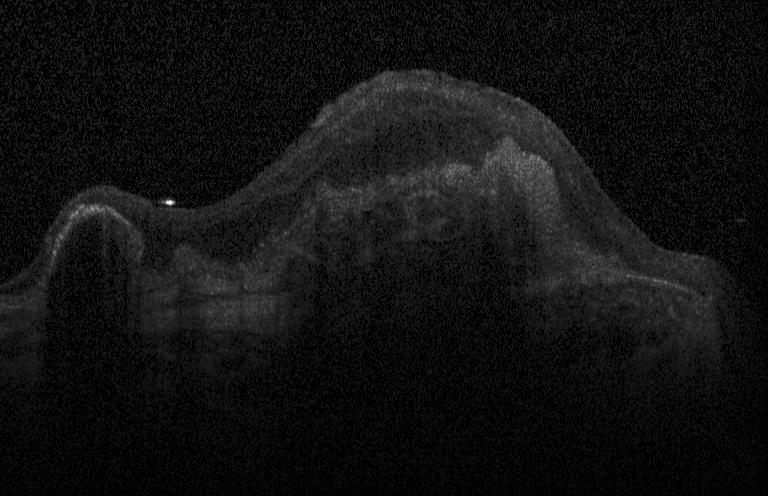 OCT finding: CNV.